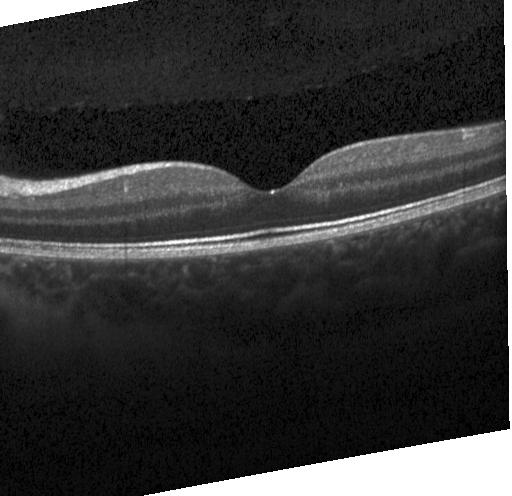

Retinal OCT B-scan
No evidence of CNV, DME, or drusen.